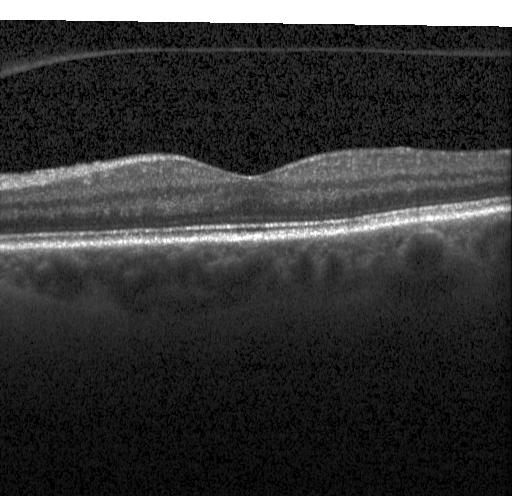 Fovea-centered · OCT B-scan.
Dx: no choroidal neovascularization, no diabetic macular edema, and no drusen.